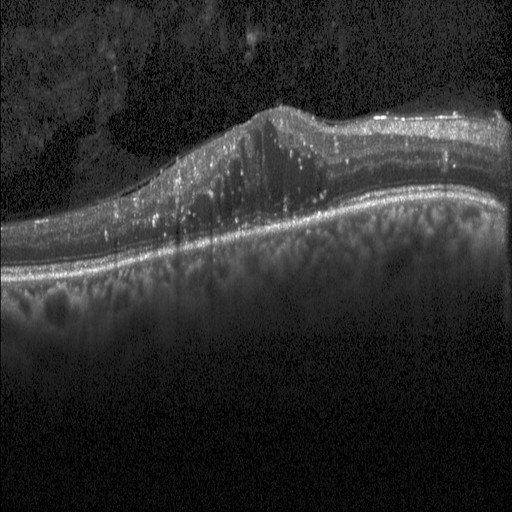
Retinal OCT cross-section, macular scan
Impression: diabetic macular edema.